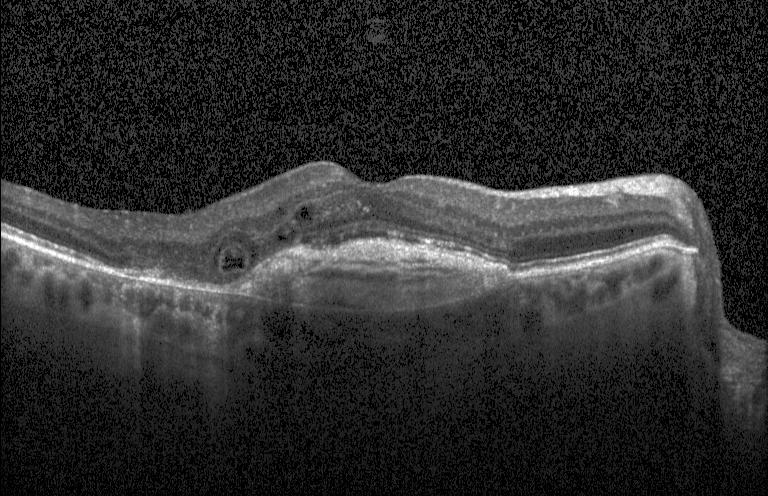

Instrument: Heidelberg Spectralis. Spectral-domain OCT. OCT B-scan. This B-scan demonstrates choroidal neovascularization.